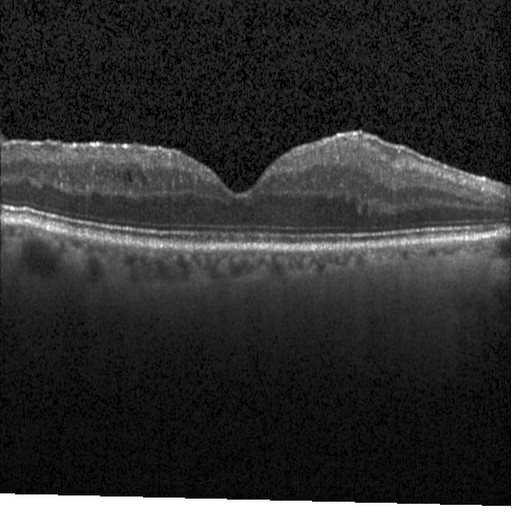
OCT line scan · spectral-domain OCT — Impression: diabetic macular edema.